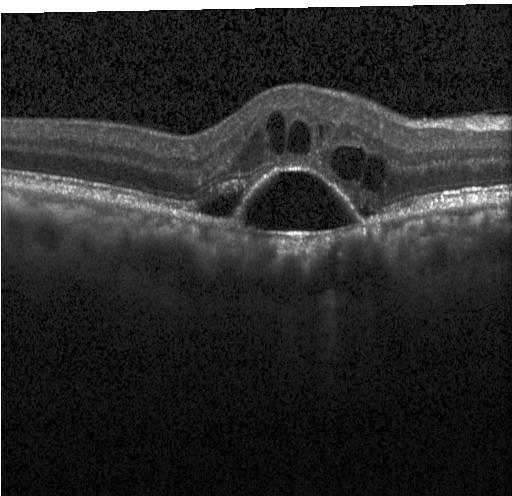

OCT B-scan · Heidelberg Spectralis.
Impression: choroidal neovascularization.